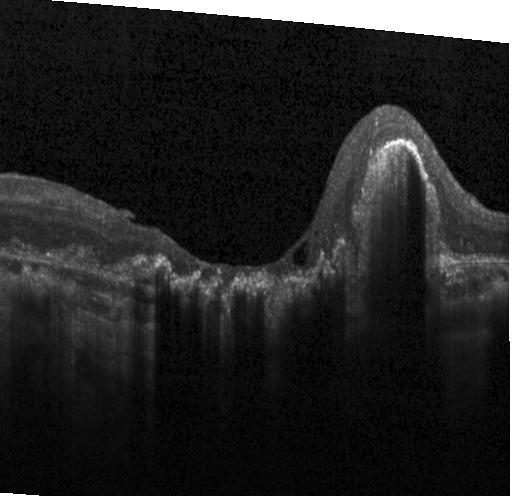
Spectral-domain optical coherence tomography · fovea-centered · acquired on a Heidelberg Spectralis · optical coherence tomography scan. Diagnosis: choroidal neovascularization (CNV).